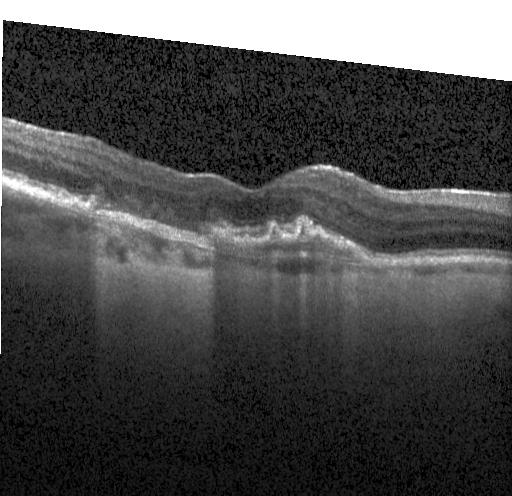

Dx: a choroidal neovascular membrane.